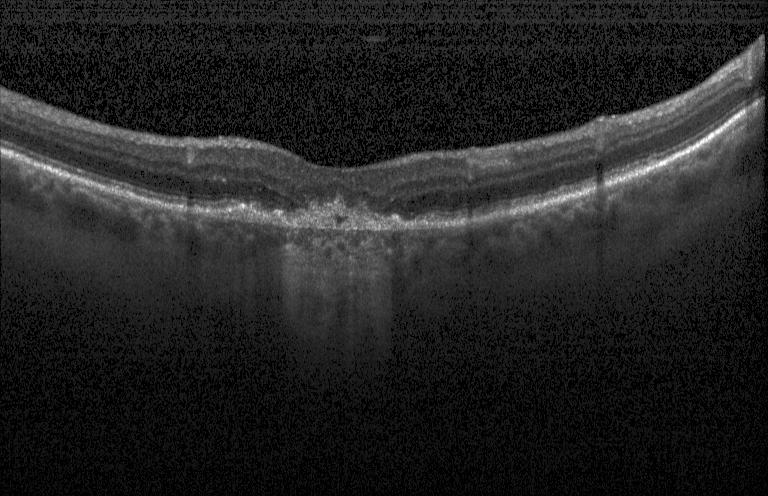
Macular scan; retinal OCT B-scan; SD-OCT. Choroidal neovascularization.